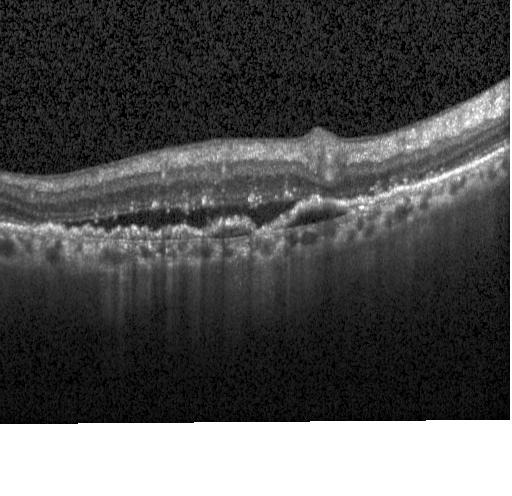
Spectral-domain OCT B-scan: a choroidal neovascular membrane.